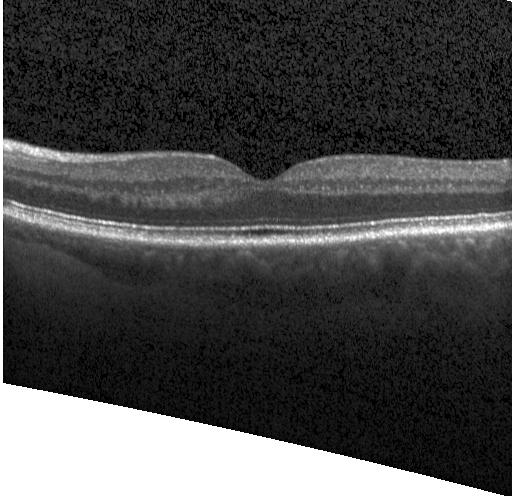 Spectral-domain OCT B-scan: no CNV, DME, or drusen.